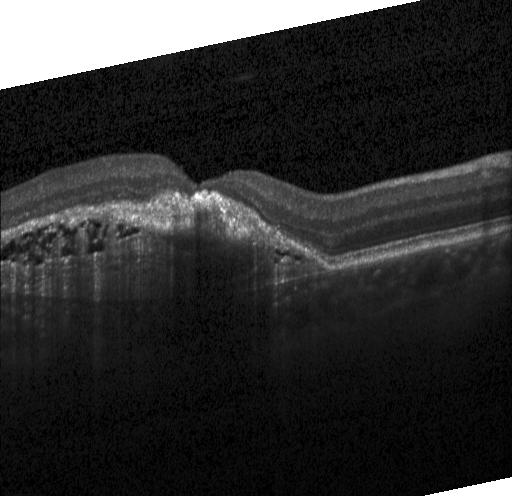 This B-scan demonstrates choroidal neovascularization (CNV).